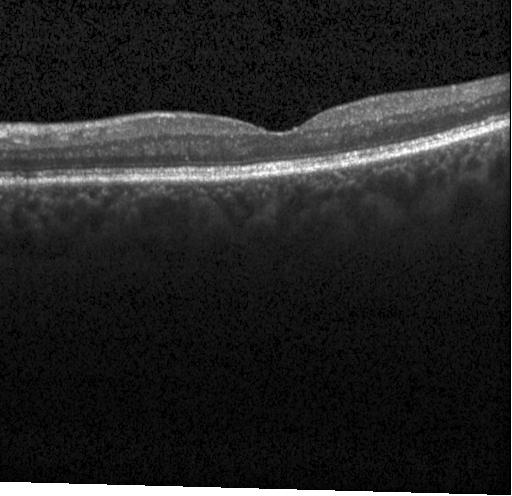
Heidelberg Spectralis OCT system; OCT B-scan; fovea-centered — OCT finding: no choroidal neovascularization, no diabetic macular edema, and no drusen.